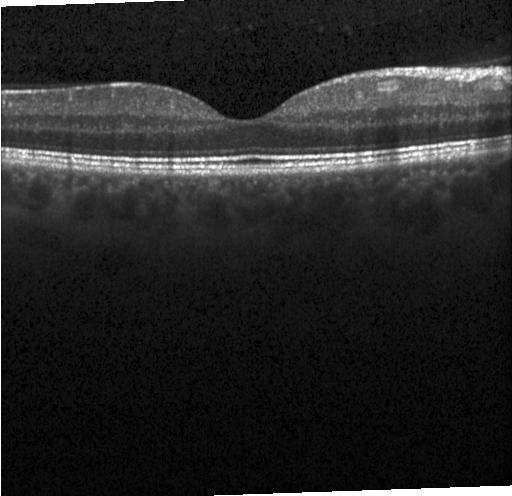

Heidelberg Spectralis, optical coherence tomography scan. Diagnosis: no choroidal neovascularization, no diabetic macular edema, and no drusen.